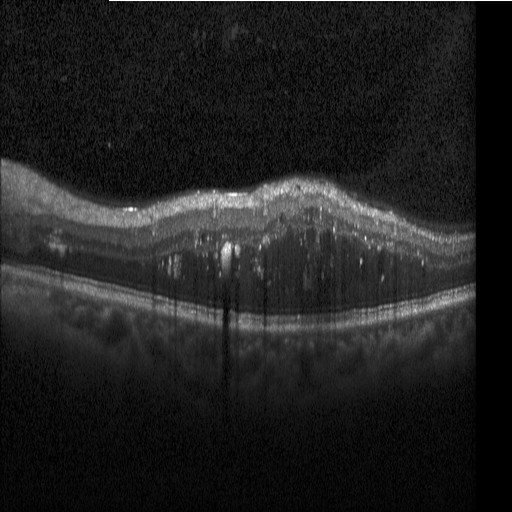
Diagnosis: diabetic macular edema (DME).